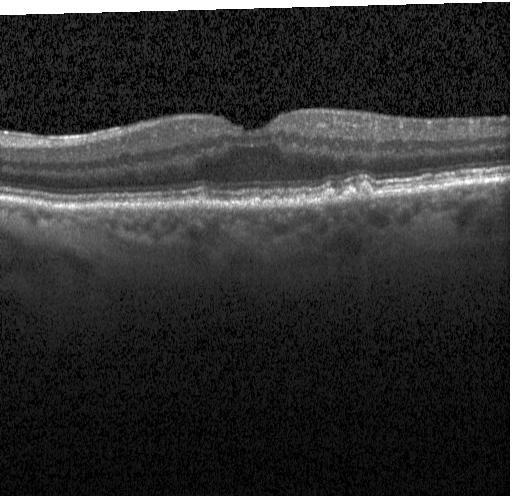
Retinal OCT cross-section, SD-OCT, Heidelberg Spectralis OCT system, macular scan. Finding: drusen.